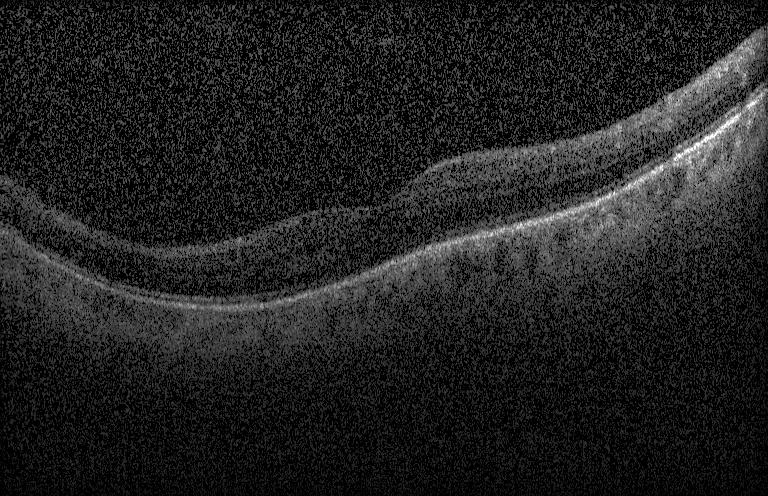

Instrument: Heidelberg Spectralis · macular scan · OCT B-scan · spectral-domain OCT.
Assessment: no CNV, no DME, and no drusen.